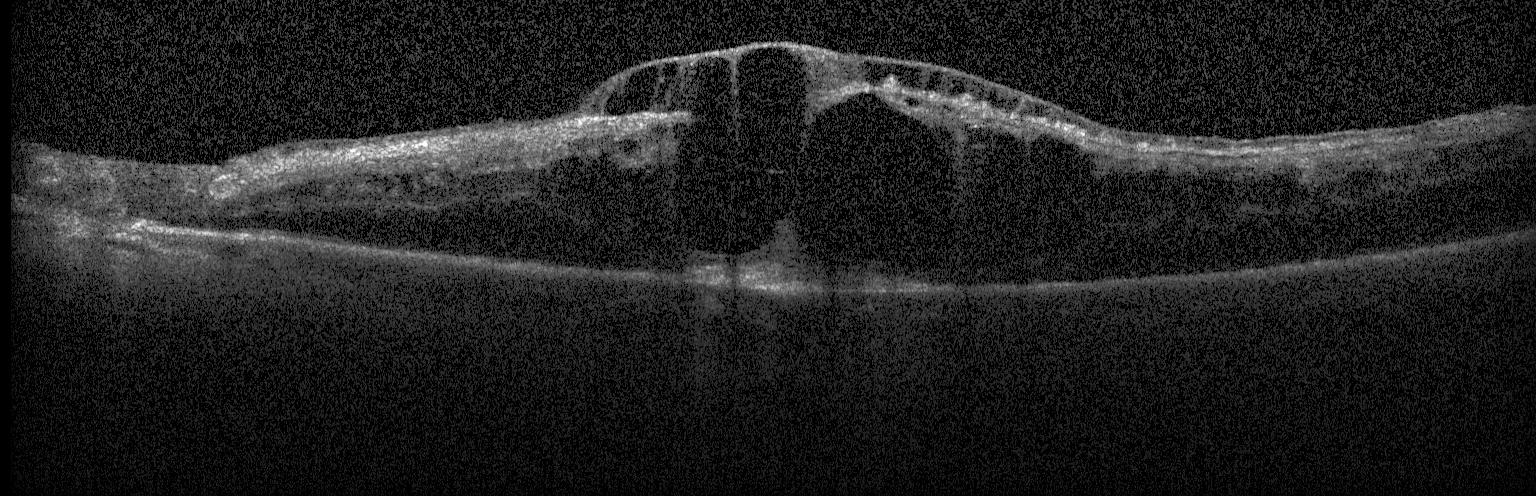

Optical coherence tomography B-scan · SD-OCT.
Finding: diabetic macular edema.